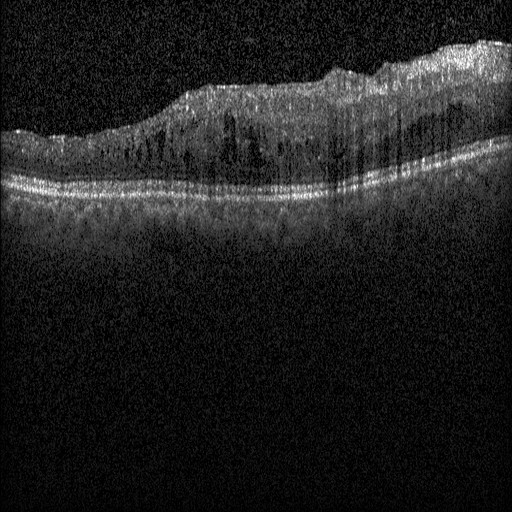
Macular OCT: diabetic macular edema (DME).